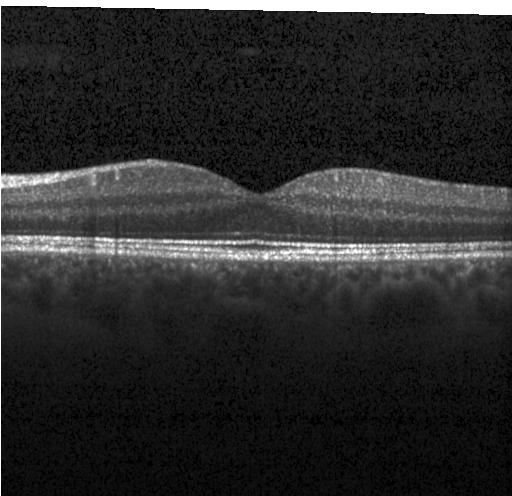

Macular OCT: no choroidal neovascularization, diabetic macular edema, or drusen.